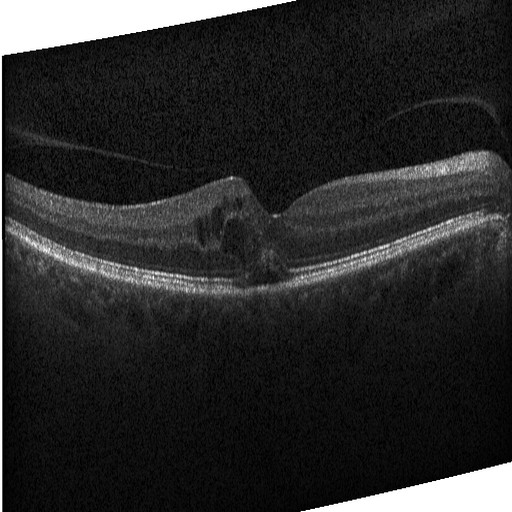 Heidelberg Spectralis OCT system; SD-OCT; horizontal scan through the fovea; retinal OCT cross-section
Diagnosis: DME.